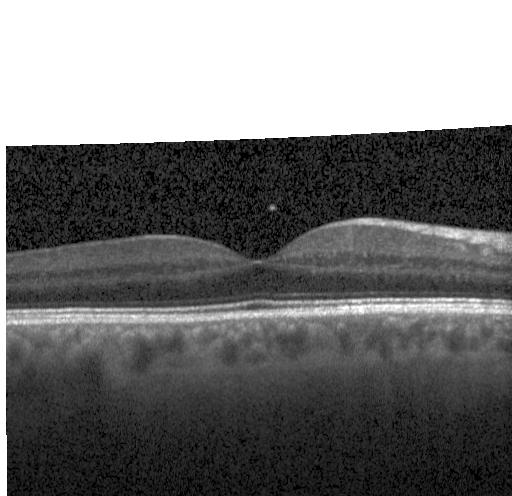 Optical coherence tomography scan · acquired on a Heidelberg Spectralis
Impression: no evidence of choroidal neovascularization, diabetic macular edema, or drusen.